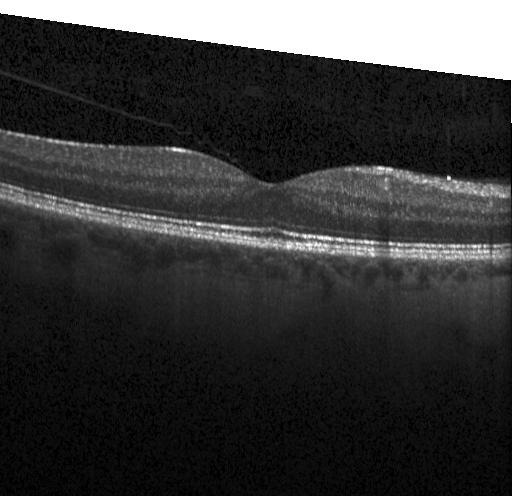 Dx: neither choroidal neovascularization, diabetic macular edema, nor drusen.